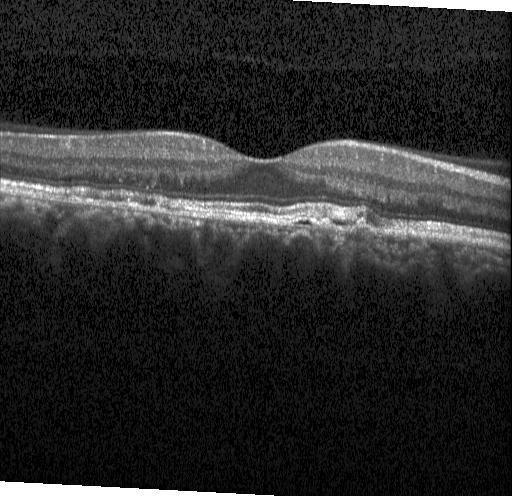 Assessment: multiple drusen.